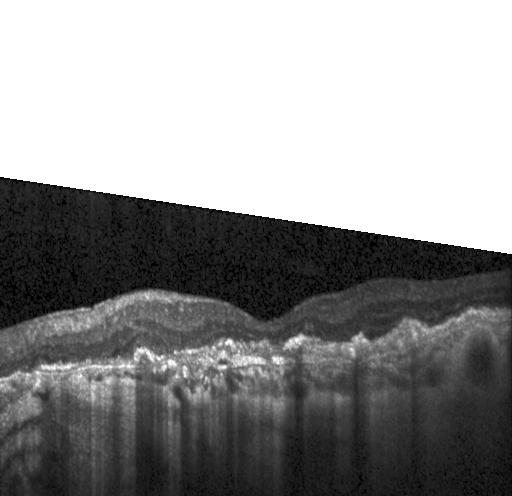 Macular OCT: choroidal neovascularization.